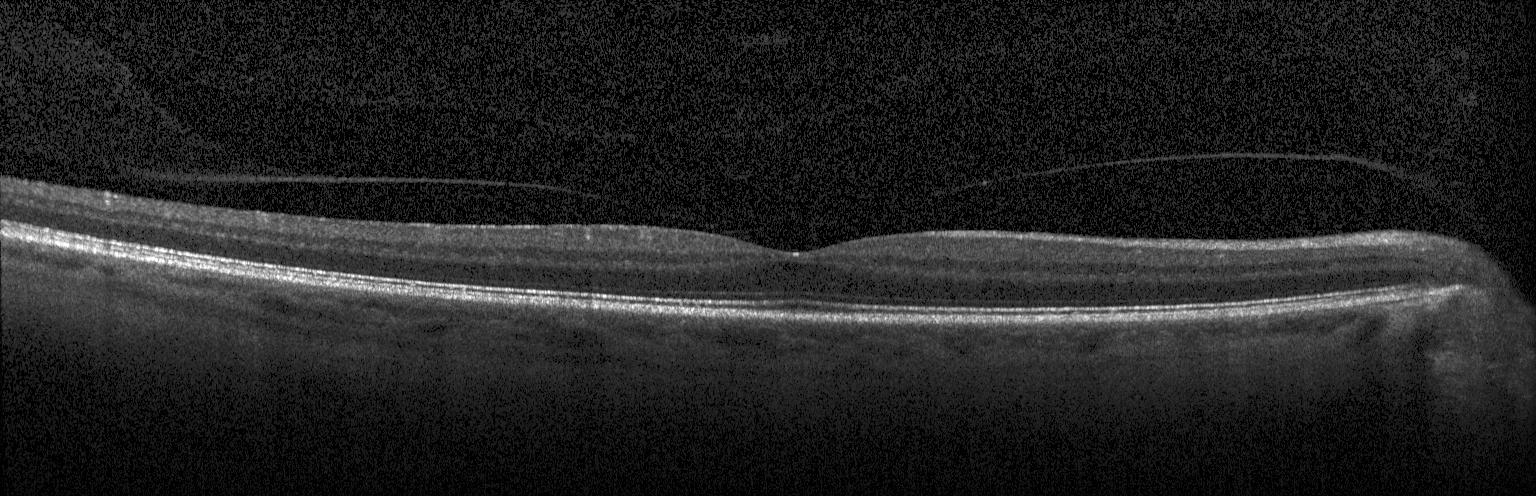

Retinal OCT cross-section
No choroidal neovascularization, diabetic macular edema, or drusen.